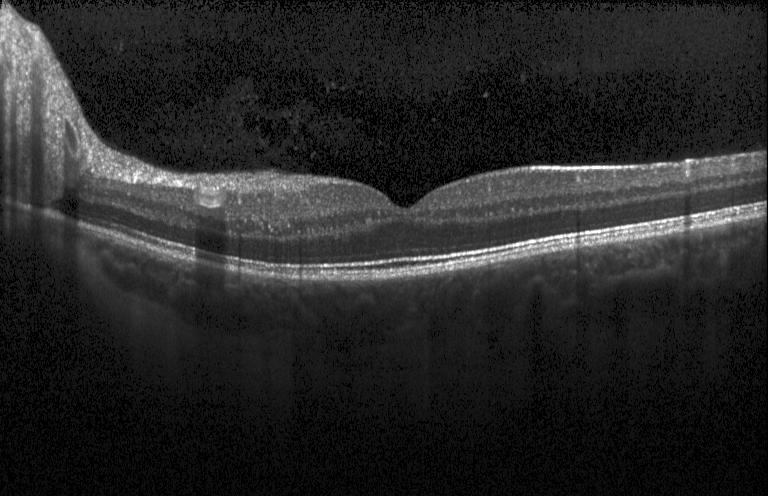 Finding: no choroidal neovascularization, diabetic macular edema, or drusen.